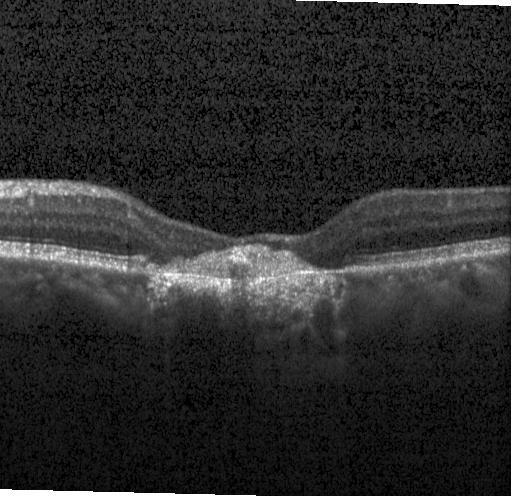
Optical coherence tomography scan.
Finding: choroidal neovascularization (CNV).